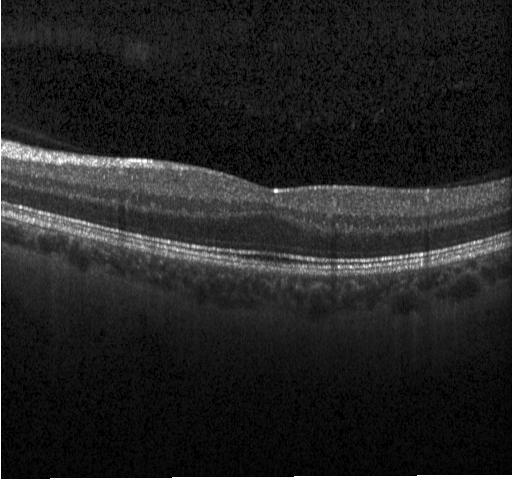 Retinal OCT B-scan; Heidelberg Spectralis; centered on the fovea; spectral-domain optical coherence tomography — Finding: no CNV, no DME, and no drusen.